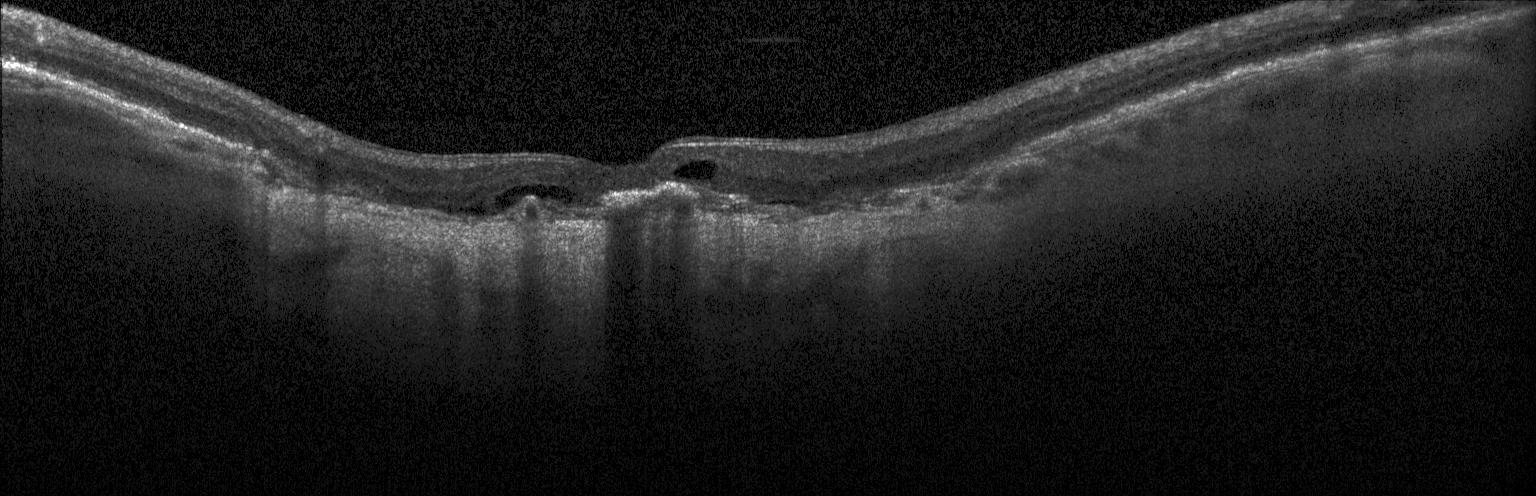
Retinal OCT cross-section showing a choroidal neovascular membrane.